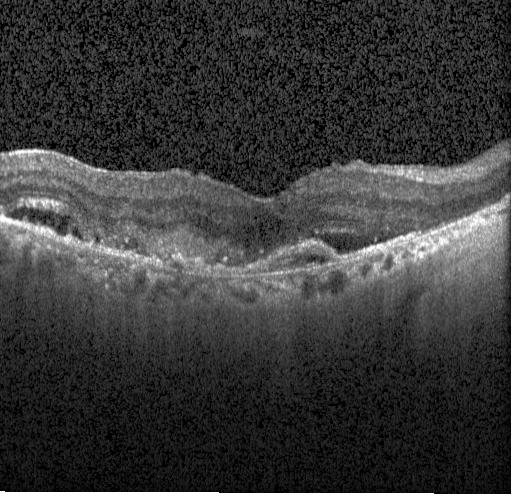
Spectral-domain OCT. Heidelberg Spectralis. Horizontal scan through the fovea. OCT B-scan
Impression: a choroidal neovascular membrane.